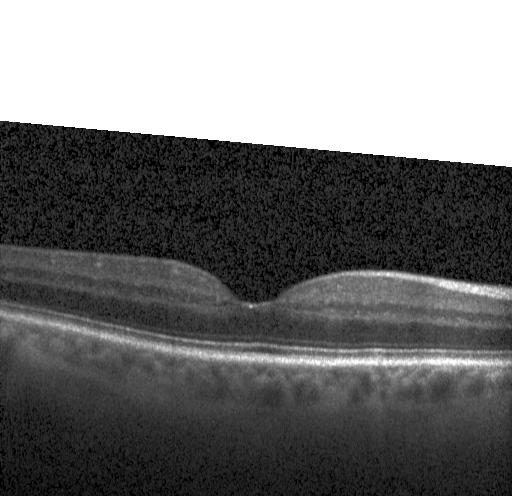 No choroidal neovascularization, diabetic macular edema, or drusen.